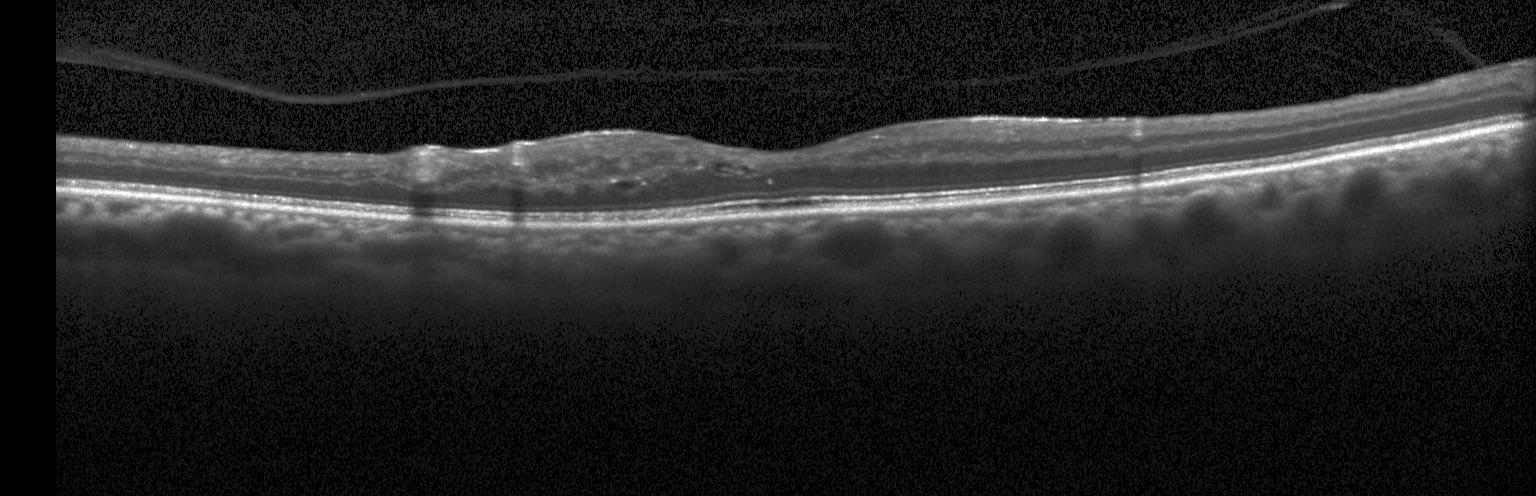

Diagnosis: diabetic macular edema (DME).